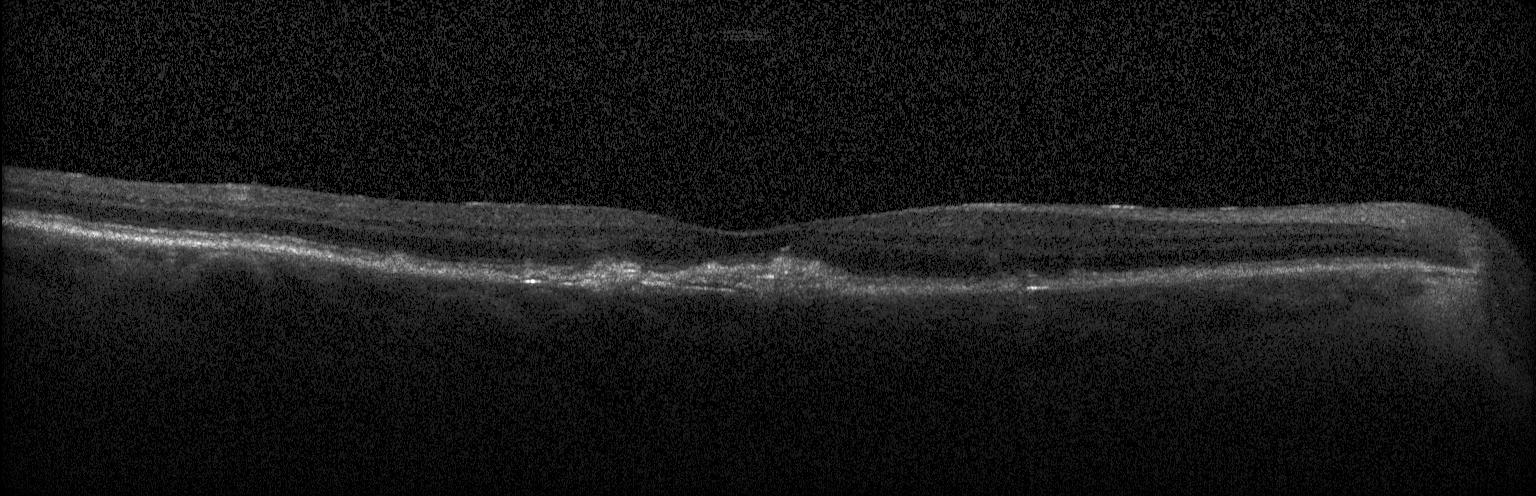

Finding: CNV.